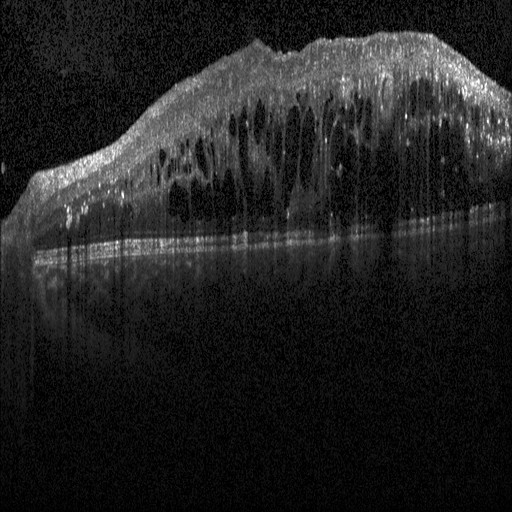

Diagnosis: diabetic macular edema.